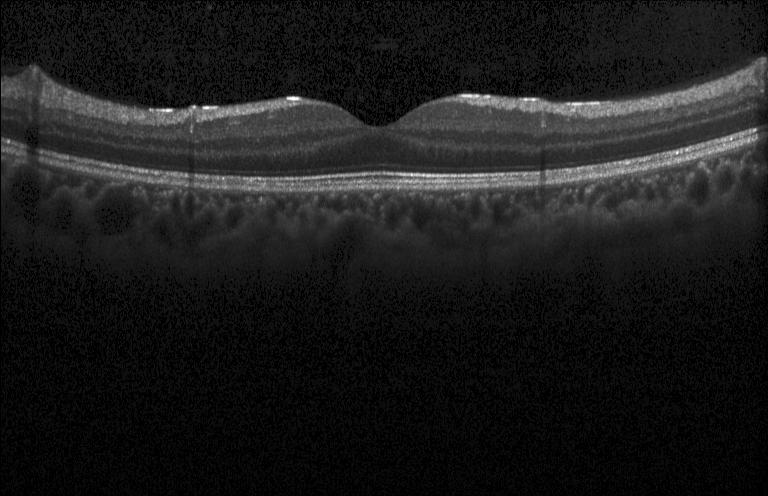 Optical coherence tomography scan. Fovea-centered. Spectral-domain optical coherence tomography — Finding: no choroidal neovascularization, diabetic macular edema, or drusen.